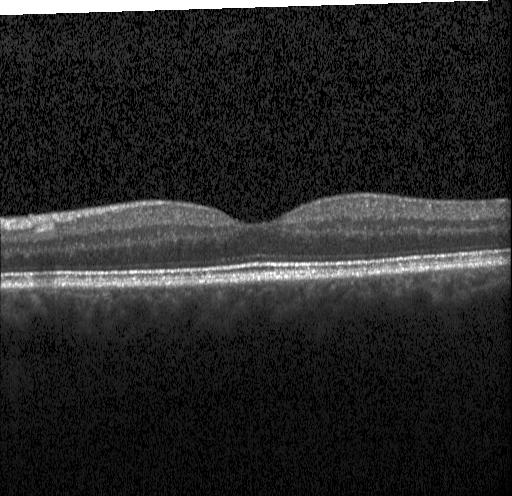 Horizontal scan through the fovea, spectral-domain optical coherence tomography, OCT line scan, Heidelberg Spectralis OCT system — Impression: no choroidal neovascularization, no diabetic macular edema, and no drusen.